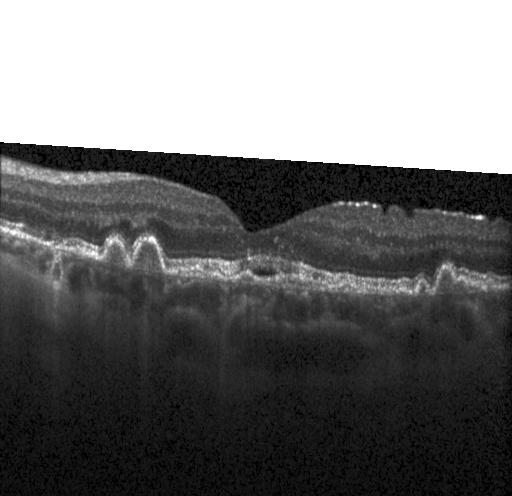
Horizontal scan through the fovea, spectral-domain OCT, acquired on a Heidelberg Spectralis, optical coherence tomography B-scan.
OCT finding: a choroidal neovascular membrane.